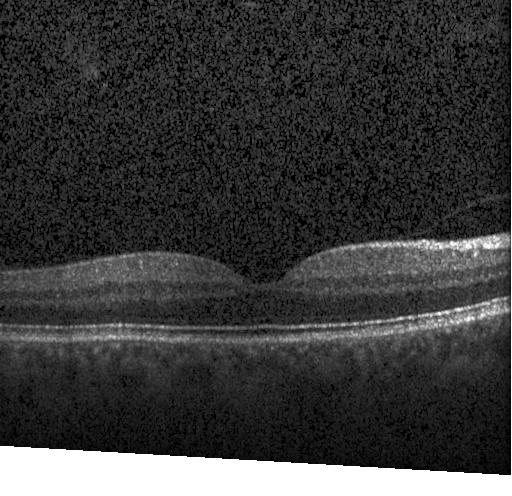

Retinal OCT cross-section; spectral-domain optical coherence tomography; acquired on a Heidelberg Spectralis
Assessment: no CNV, DME, or drusen.